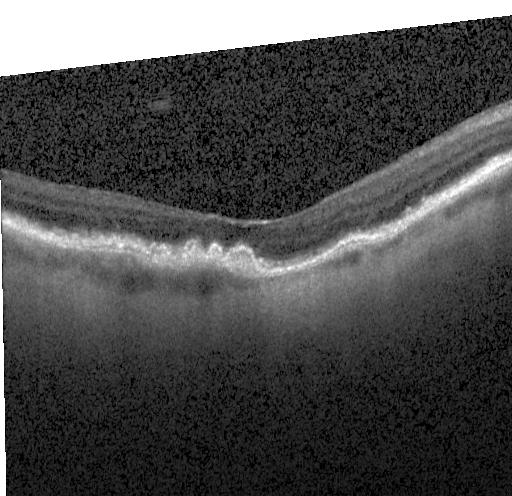

Acquired on a Heidelberg Spectralis. Spectral-domain optical coherence tomography. OCT B-scan. Centered on the fovea
Finding: a choroidal neovascular membrane.